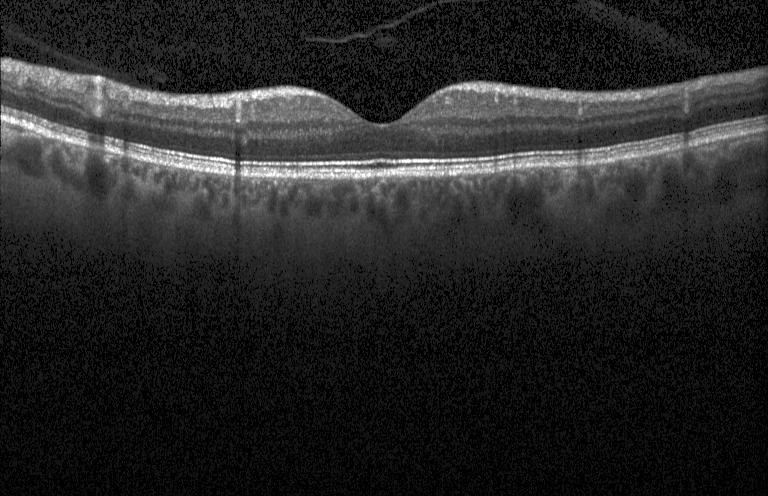

Impression: no choroidal neovascularization, no diabetic macular edema, and no drusen.